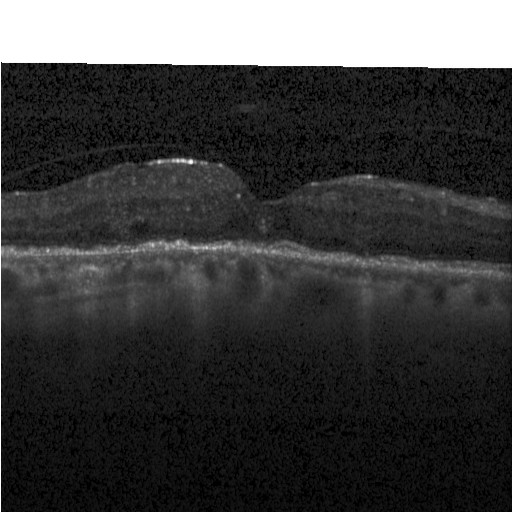 OCT scan showing diabetic macular edema (DME).